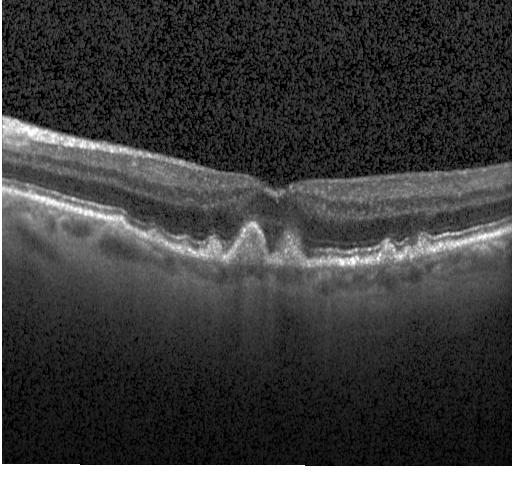 Diagnosis: multiple drusen.